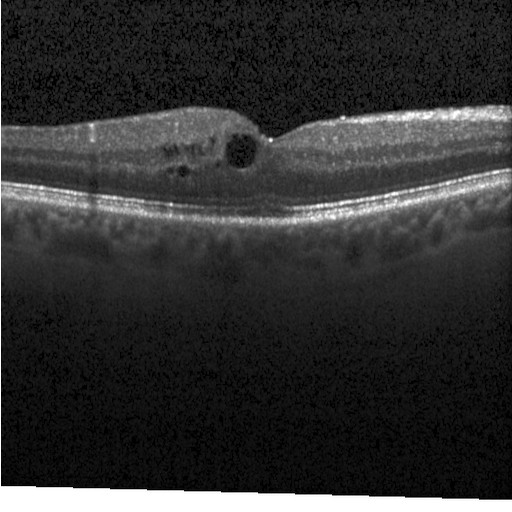

OCT B-scan. Instrument: Heidelberg Spectralis. Spectral-domain optical coherence tomography — Finding: diabetic macular edema.